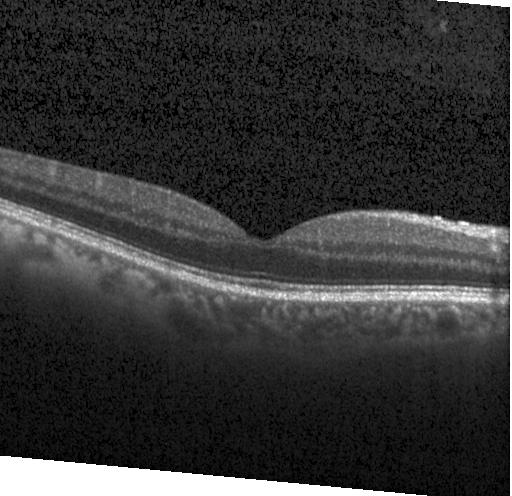 Instrument: Heidelberg Spectralis. Centered on the fovea. Retinal OCT B-scan — No evidence of CNV, DME, or drusen.